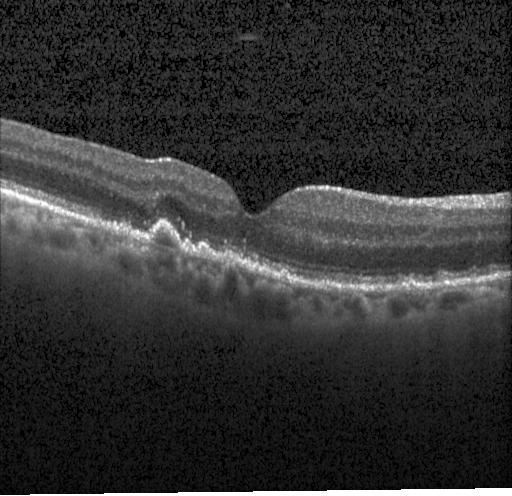
Retinal OCT B-scan, Heidelberg Spectralis
Impression: multiple drusen.